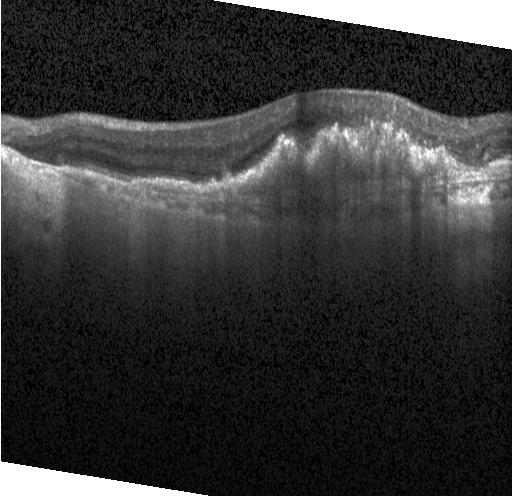 Fovea-centered; optical coherence tomography scan; Heidelberg Spectralis; spectral-domain optical coherence tomography.
Diagnosis: a choroidal neovascular membrane.